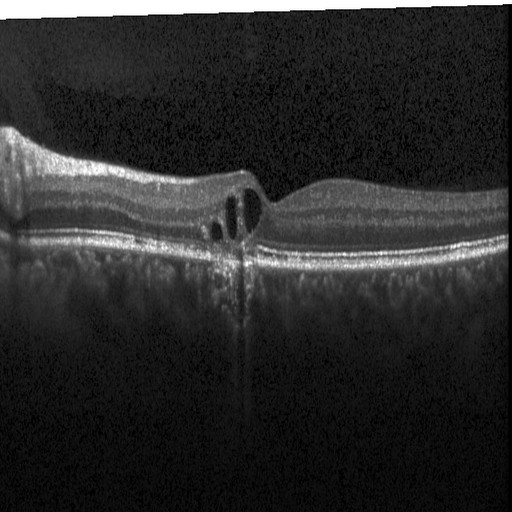

Spectral-domain optical coherence tomography · optical coherence tomography scan
Macular OCT: diabetic macular edema (DME).